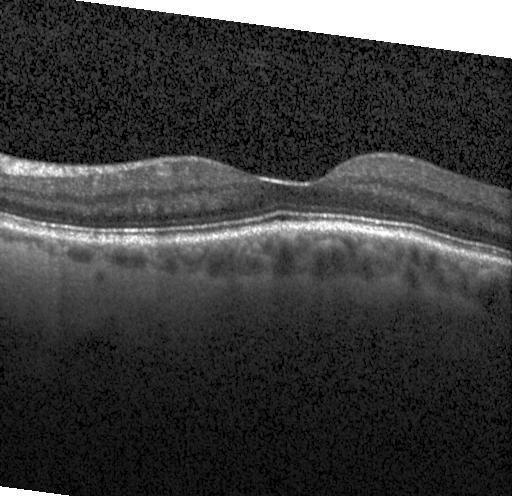

This B-scan demonstrates no evidence of choroidal neovascularization, diabetic macular edema, or drusen.